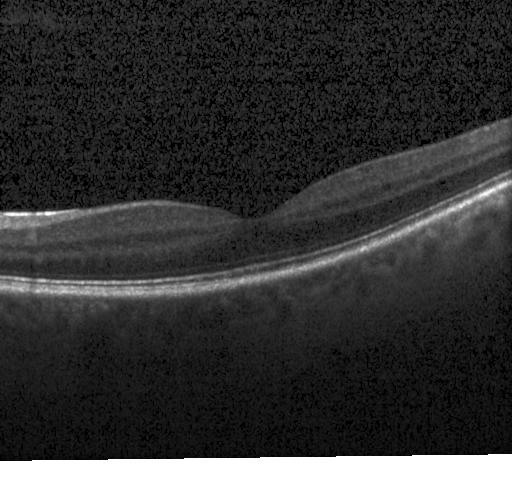
OCT B-scan
Assessment: neither choroidal neovascularization, diabetic macular edema, nor drusen.